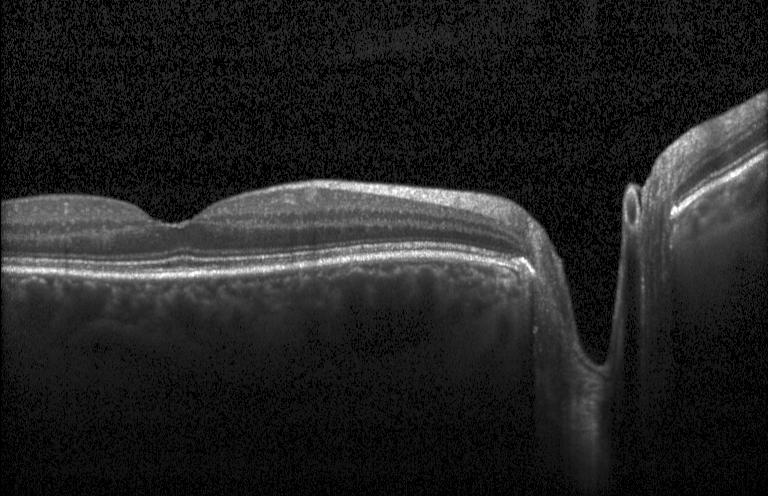 Impression: no evidence of choroidal neovascularization, diabetic macular edema, or drusen.